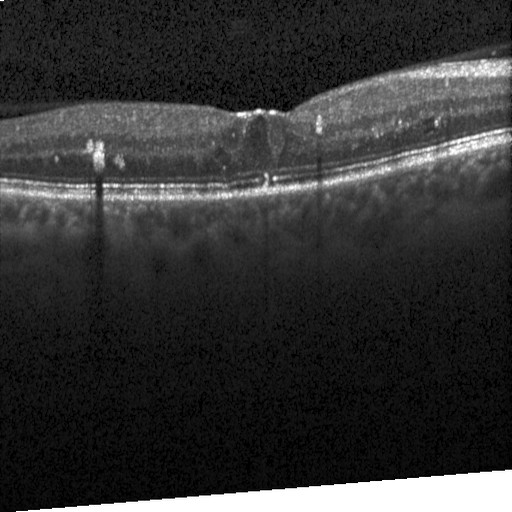 OCT B-scan showing DME.